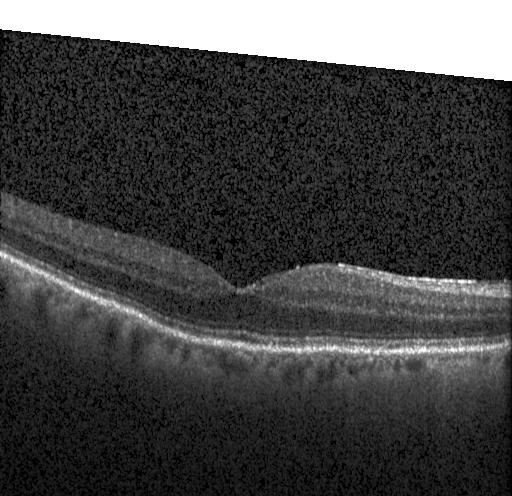

Acquired on a Heidelberg Spectralis · optical coherence tomography scan — OCT finding: no choroidal neovascularization, no diabetic macular edema, and no drusen.